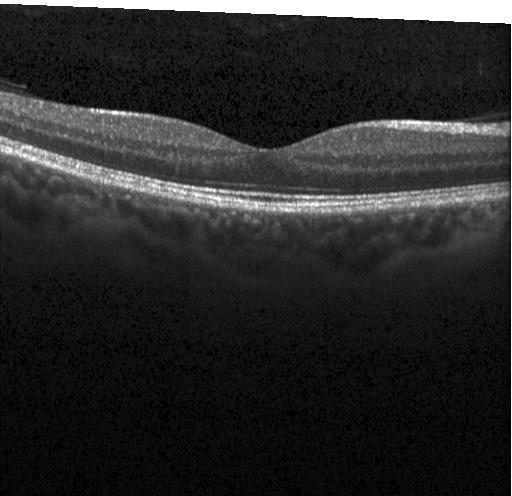 Optical coherence tomography B-scan — Assessment: no choroidal neovascularization, diabetic macular edema, or drusen.